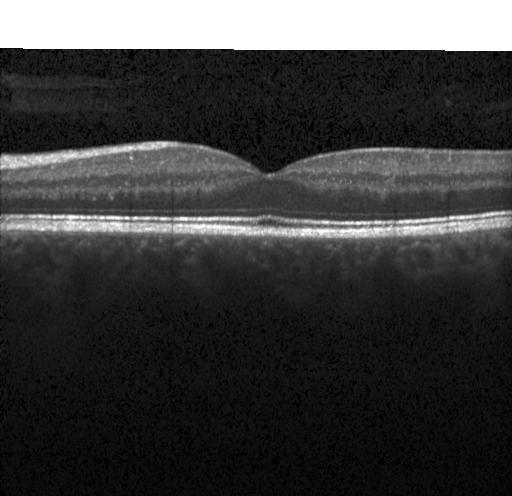

Assessment: no choroidal neovascularization, no diabetic macular edema, and no drusen.